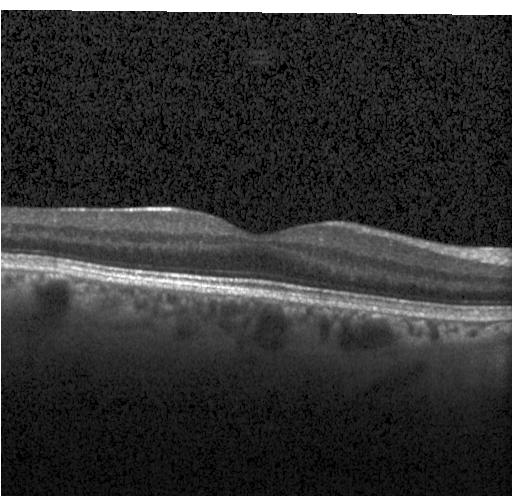 Spectral-domain OCT. Heidelberg Spectralis OCT system. Optical coherence tomography scan. Macular scan — Impression: no evidence of choroidal neovascularization, diabetic macular edema, or drusen.